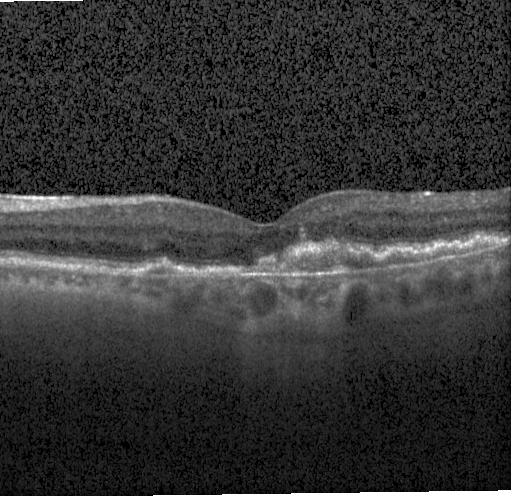
Instrument: Heidelberg Spectralis; optical coherence tomography scan
Impression: a choroidal neovascular membrane.